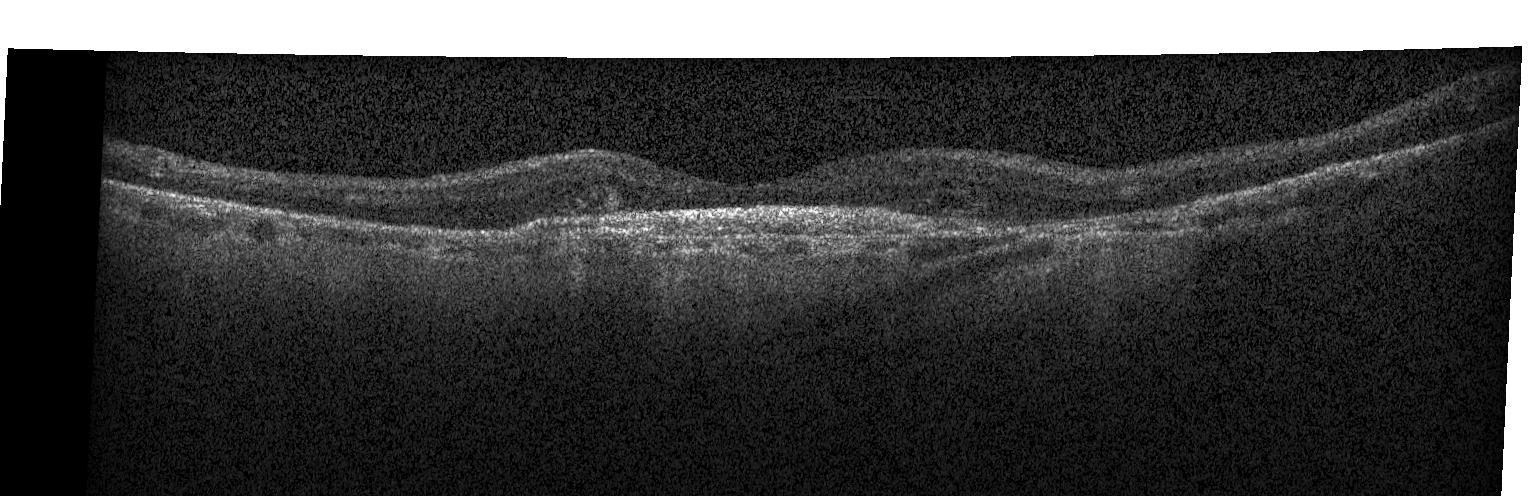
Optical coherence tomography B-scan; acquired on a Heidelberg Spectralis; horizontal scan through the fovea; spectral-domain optical coherence tomography. Impression: a choroidal neovascular membrane.